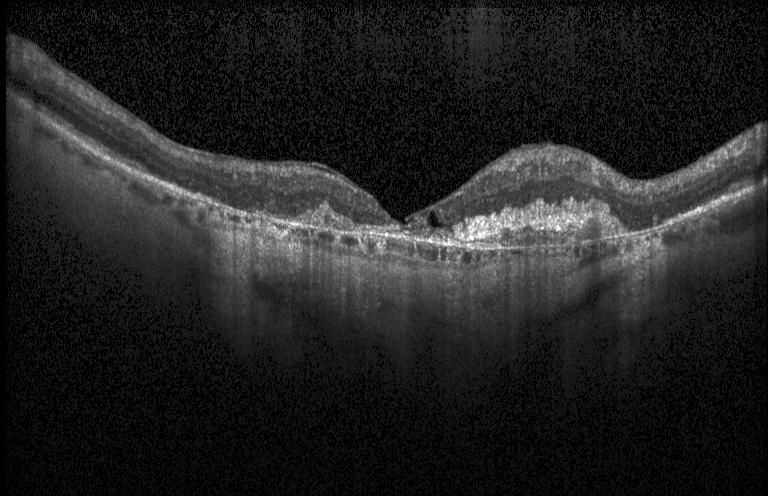

OCT B-scan — The scan shows a choroidal neovascular membrane.